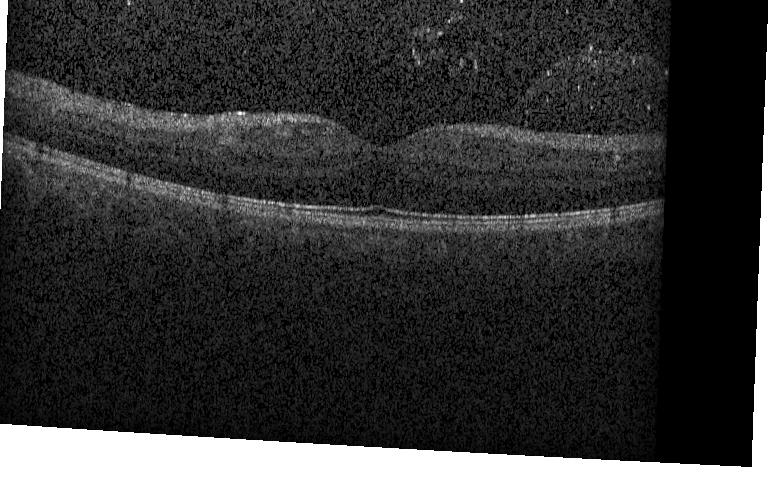

Retinal OCT cross-section, instrument: Heidelberg Spectralis.
Finding: no evidence of choroidal neovascularization, diabetic macular edema, or drusen.